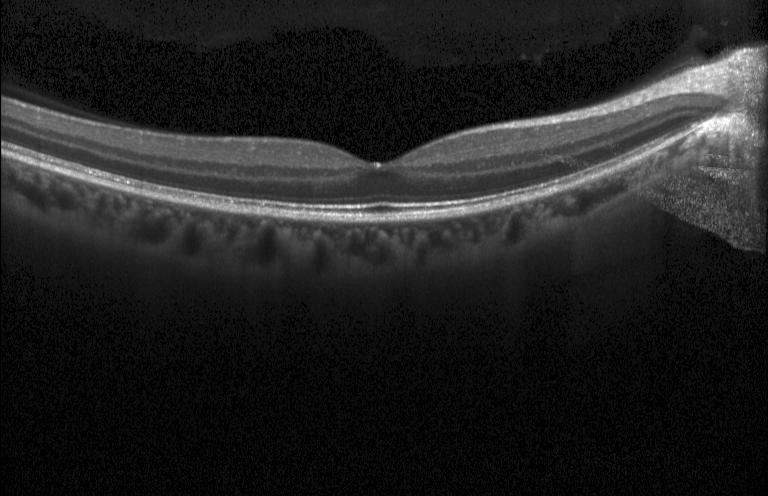
OCT line scan.
No CNV, no DME, and no drusen.